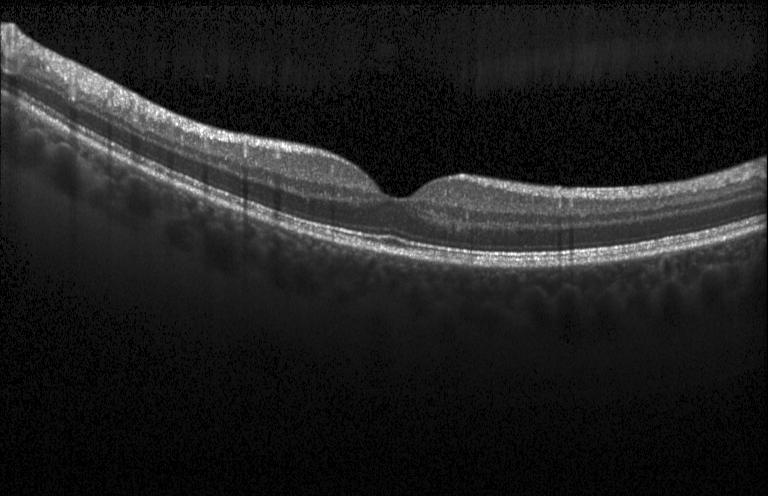
SD-OCT · OCT B-scan · macular scan. Macular OCT: neither CNV, DME, nor drusen.